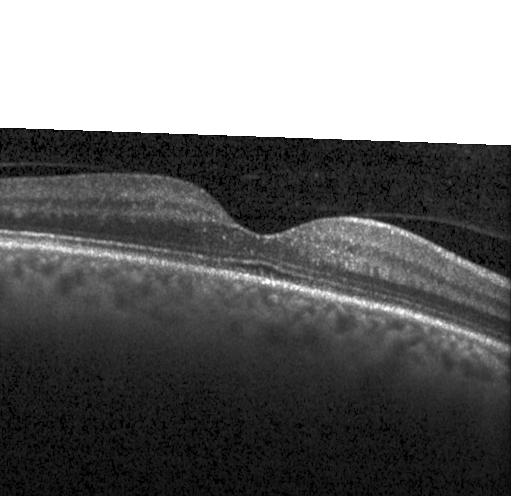

Heidelberg Spectralis · retinal OCT B-scan. Impression: no choroidal neovascularization, diabetic macular edema, or drusen.